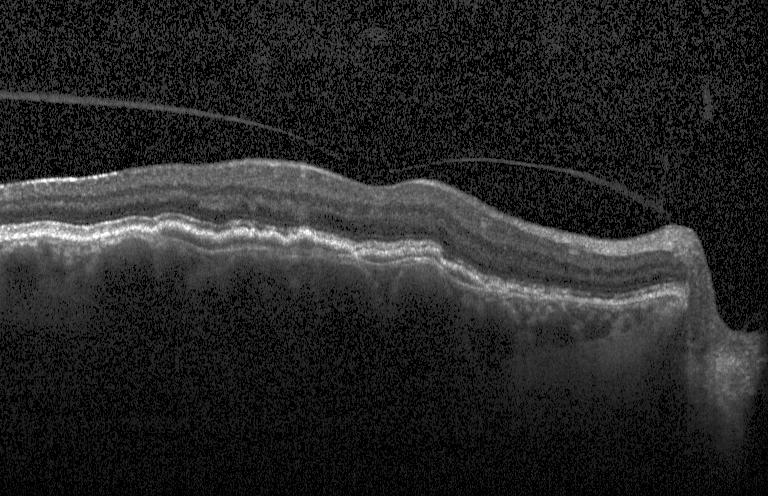
Optical coherence tomography scan. Spectral-domain optical coherence tomography. Heidelberg Spectralis — This B-scan demonstrates CNV.